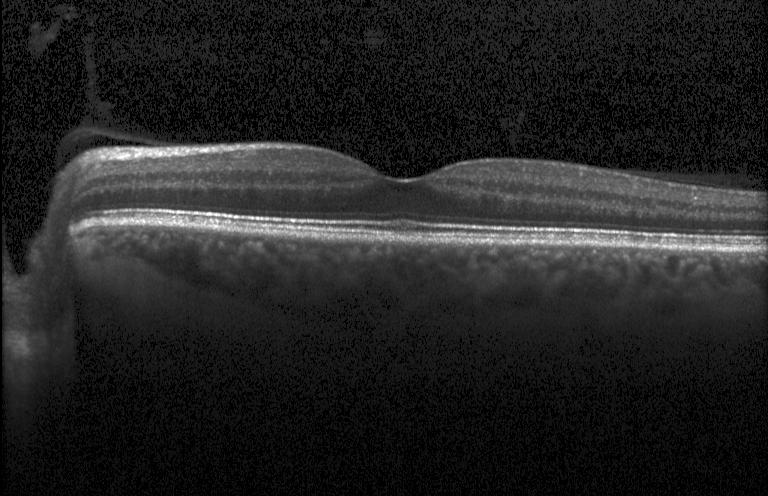

OCT line scan · instrument: Heidelberg Spectralis · centered on the fovea · SD-OCT
No choroidal neovascularization, no diabetic macular edema, and no drusen.